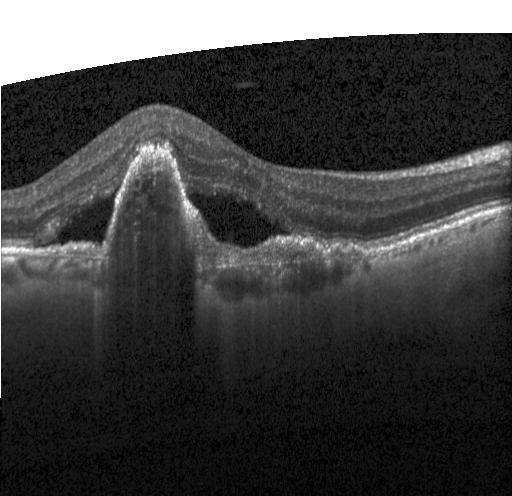 Acquired on a Heidelberg Spectralis, spectral-domain optical coherence tomography, macular scan, optical coherence tomography scan — Assessment: a choroidal neovascular membrane.